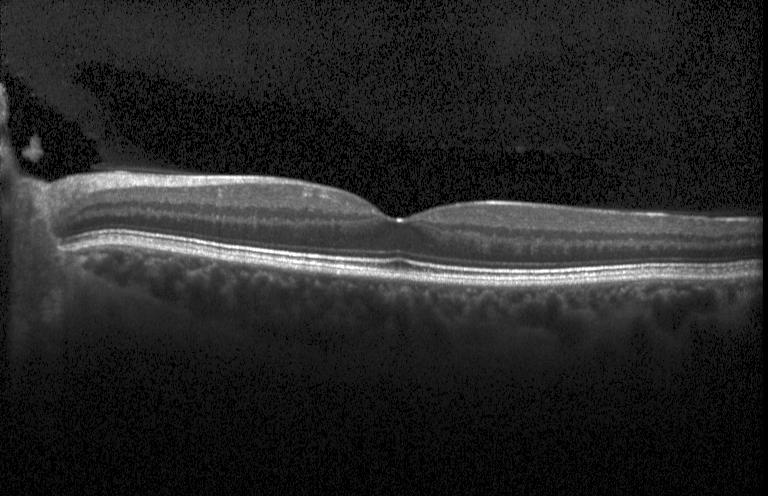 SD-OCT, optical coherence tomography B-scan.
Finding: no evidence of choroidal neovascularization, diabetic macular edema, or drusen.